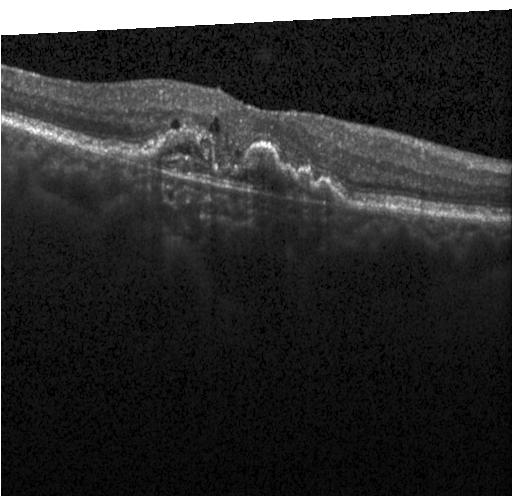
OCT B-scan. Spectral-domain OCT. Fovea-centered.
The scan shows choroidal neovascularization.